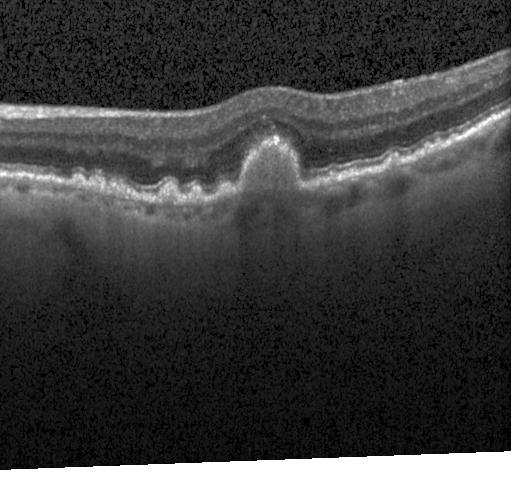 Optical coherence tomography scan — Assessment: multiple drusen.